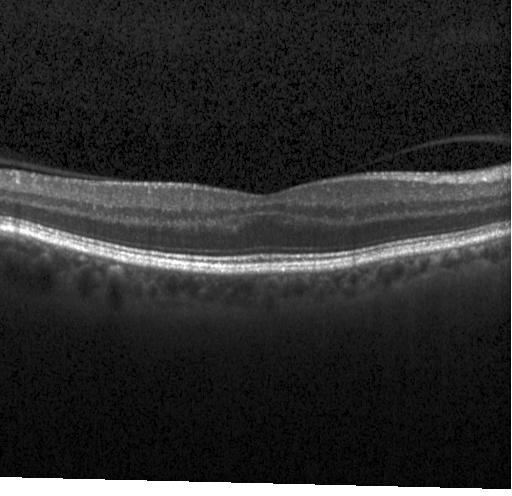

Spectral-domain OCT. Acquired on a Heidelberg Spectralis. OCT B-scan — Finding: no choroidal neovascularization, diabetic macular edema, or drusen.